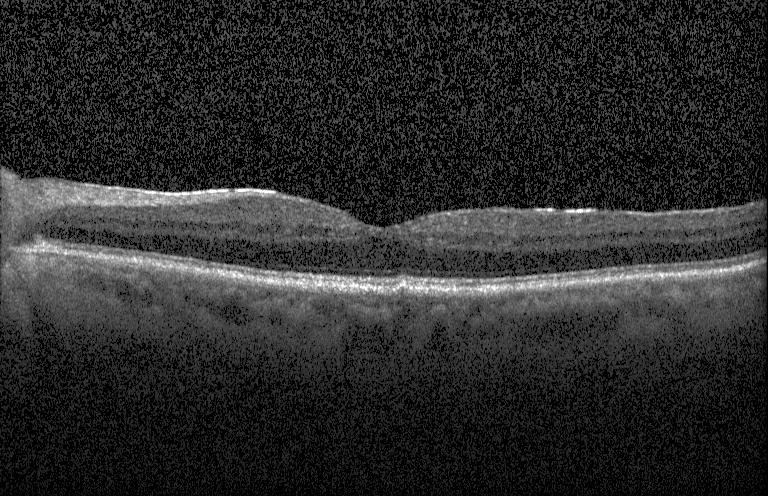

Optical coherence tomography scan — Macular OCT: neither choroidal neovascularization, diabetic macular edema, nor drusen.